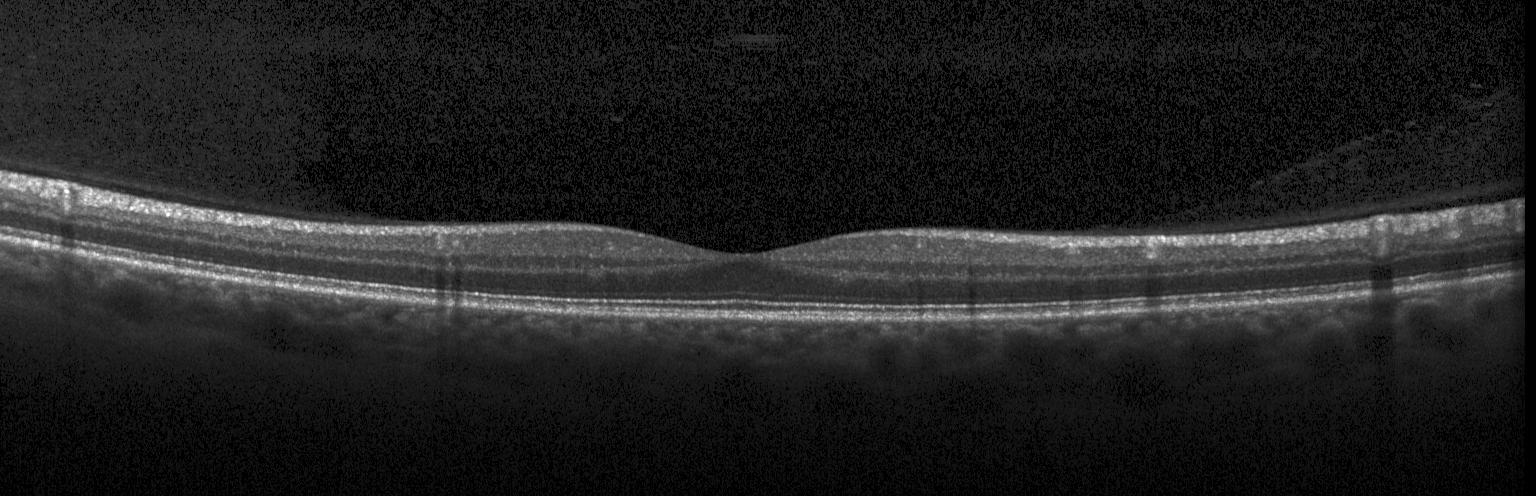

Heidelberg Spectralis. Macular scan. SD-OCT. Optical coherence tomography scan — Dx: no choroidal neovascularization, diabetic macular edema, or drusen.